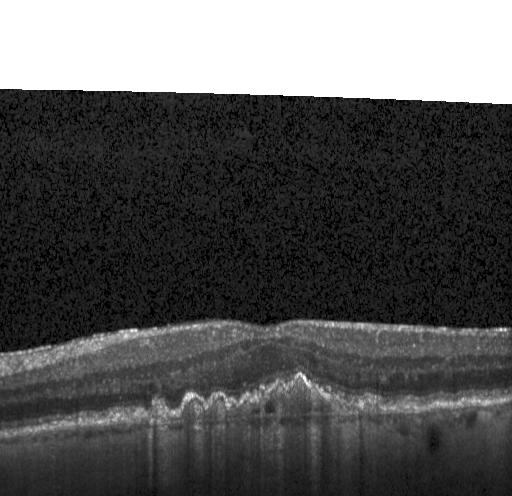 Retinal OCT B-scan, Heidelberg Spectralis OCT system, spectral-domain optical coherence tomography. Assessment: a choroidal neovascular membrane.